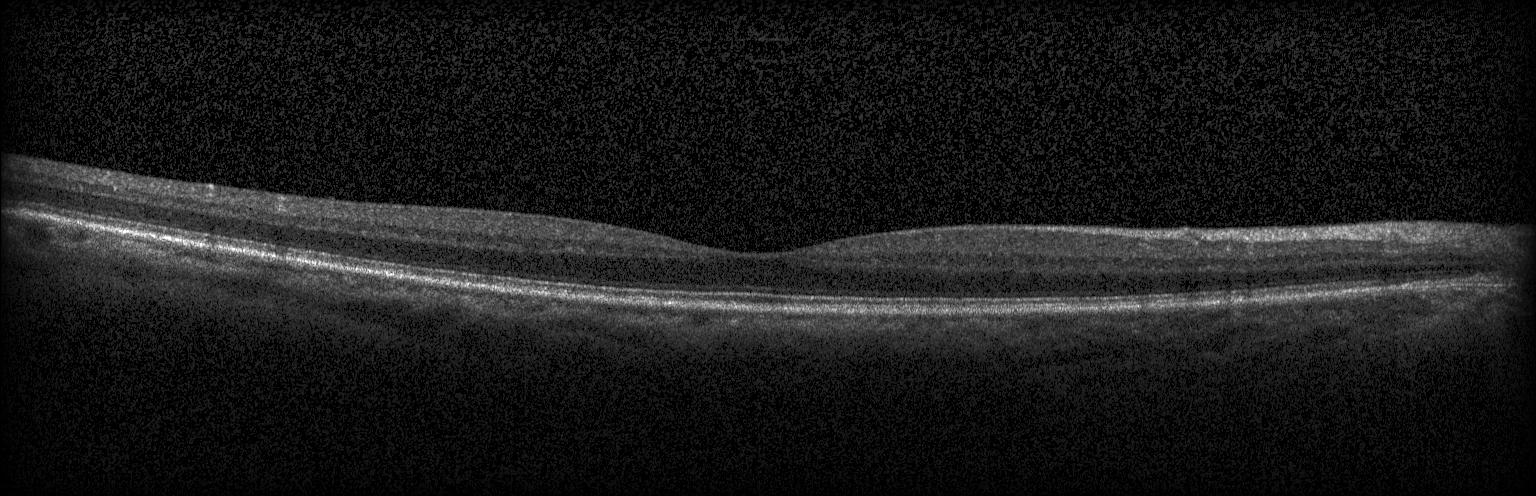 SD-OCT. OCT line scan. Macular OCT: neither choroidal neovascularization, diabetic macular edema, nor drusen.